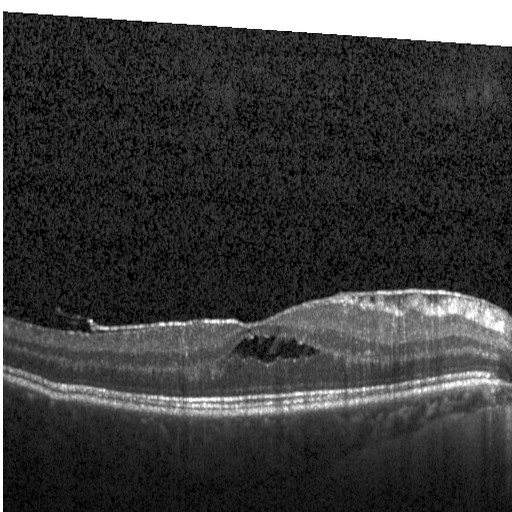
Finding: DME.